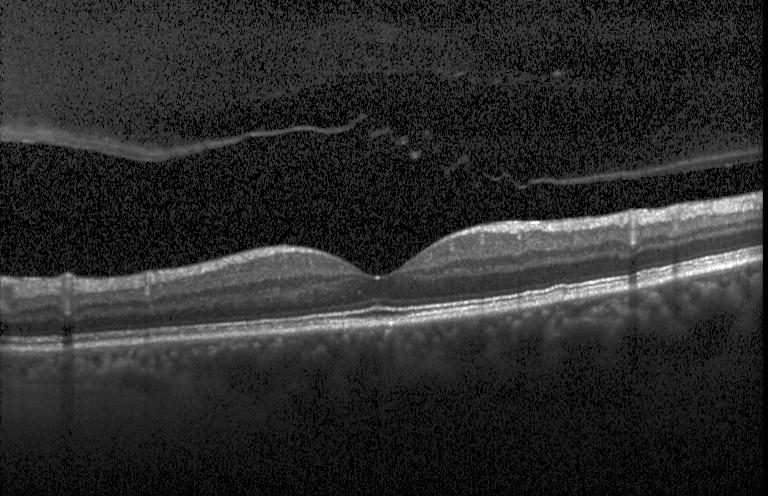
OCT line scan.
Assessment: no choroidal neovascularization, no diabetic macular edema, and no drusen.